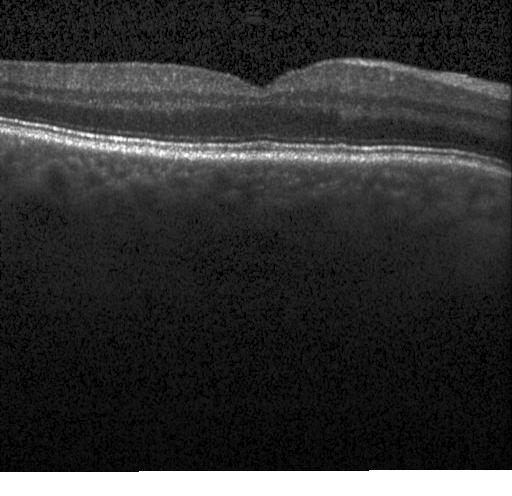 Spectral-domain OCT. Optical coherence tomography scan.
Finding: neither CNV, DME, nor drusen.